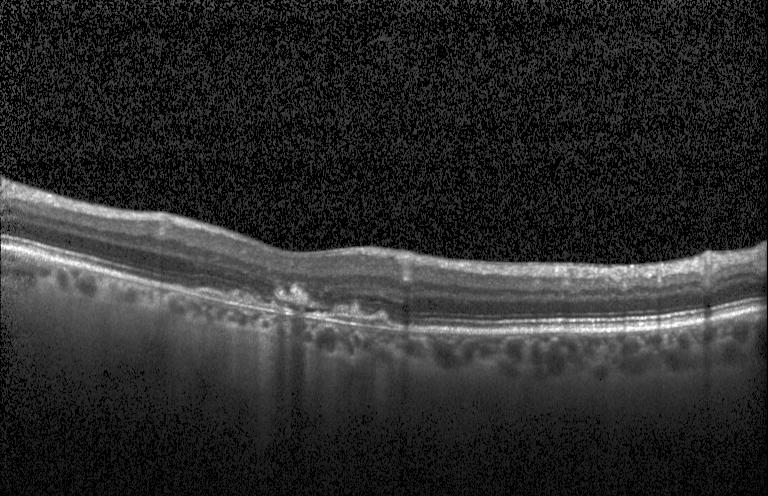

Dx: a choroidal neovascular membrane.